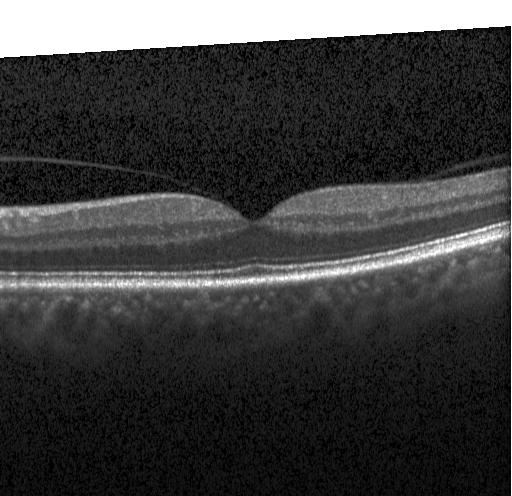 Macular OCT: no choroidal neovascularization, diabetic macular edema, or drusen.